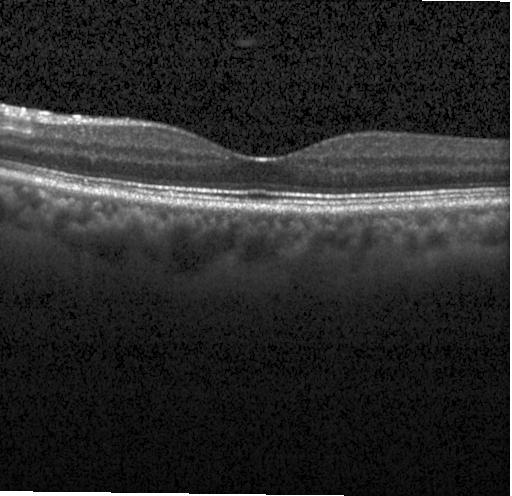
Macular OCT: no choroidal neovascularization, no diabetic macular edema, and no drusen.